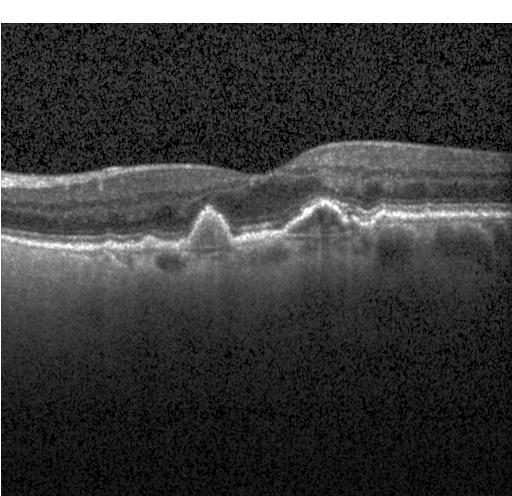
Macular scan · spectral-domain optical coherence tomography · instrument: Heidelberg Spectralis · OCT B-scan
Finding: a choroidal neovascular membrane.